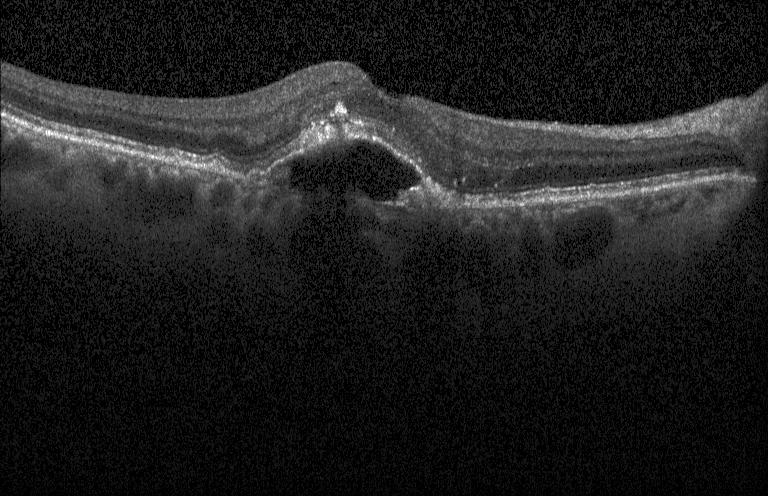
Instrument: Heidelberg Spectralis, optical coherence tomography B-scan, macular scan.
The scan shows a choroidal neovascular membrane.